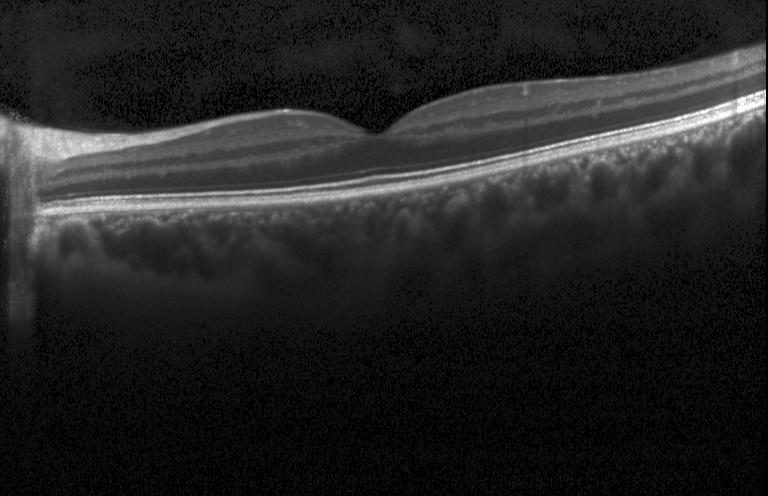 Spectral-domain OCT; retinal OCT B-scan. Diagnosis: neither choroidal neovascularization, diabetic macular edema, nor drusen.